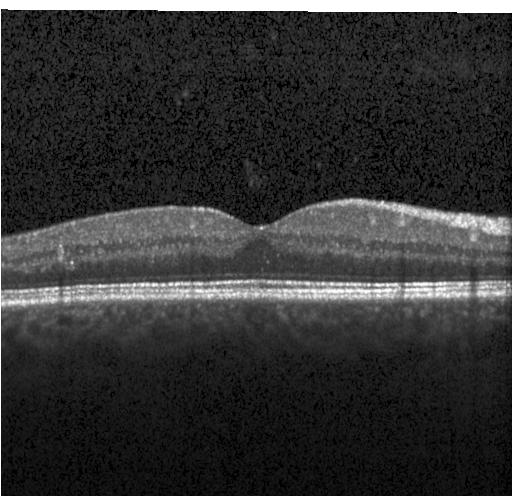
Optical coherence tomography scan, acquired on a Heidelberg Spectralis, through the macula, spectral-domain OCT. Diagnosis: neither choroidal neovascularization, diabetic macular edema, nor drusen.